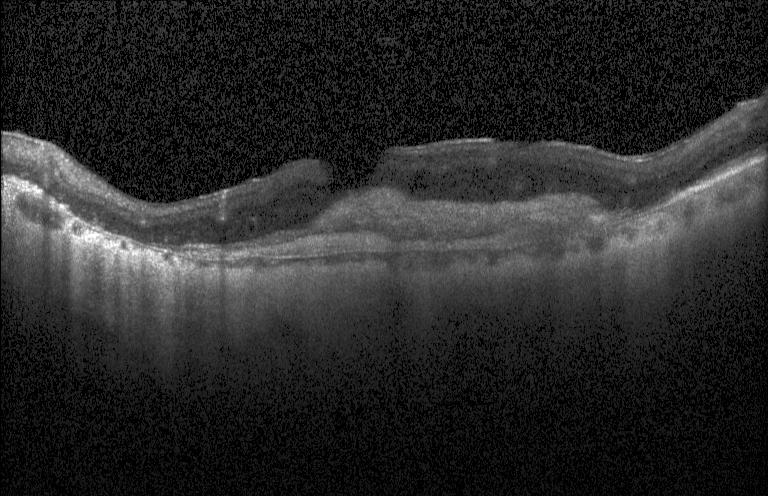

Retinal OCT cross-section.
Diagnosis: a choroidal neovascular membrane.